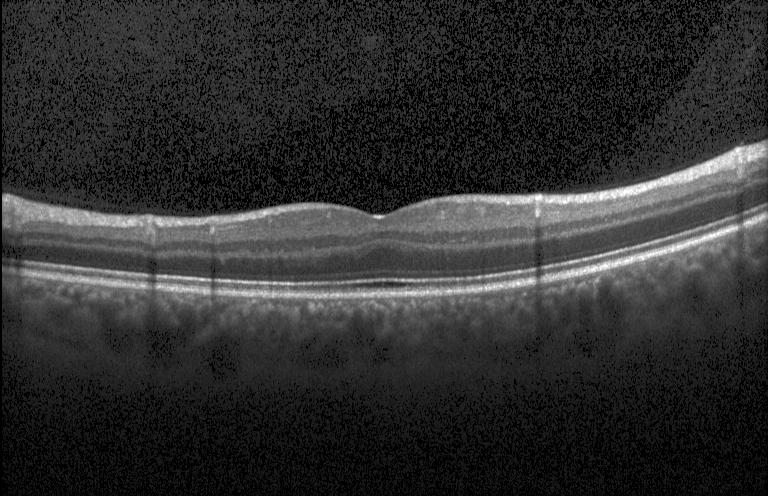 Retinal OCT B-scan — The scan shows no choroidal neovascularization, no diabetic macular edema, and no drusen.